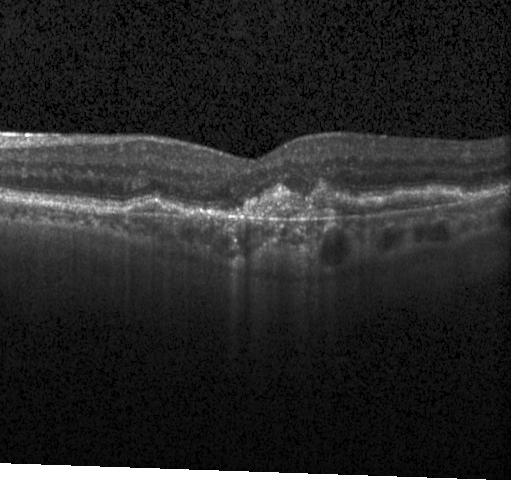 Optical coherence tomography scan · through the macula — Macular OCT: a choroidal neovascular membrane.